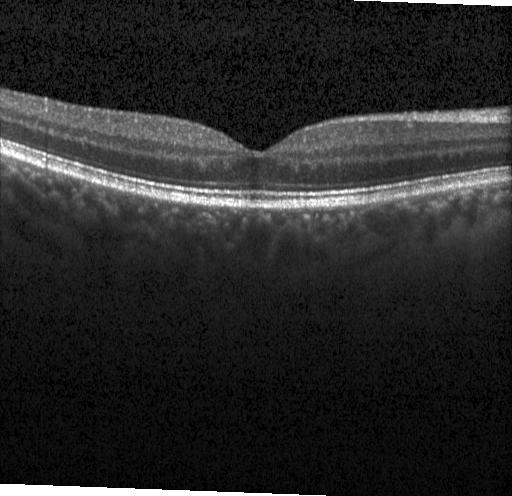

Retinal OCT B-scan. Through the macula. Instrument: Heidelberg Spectralis. Diagnosis: no CNV, no DME, and no drusen.